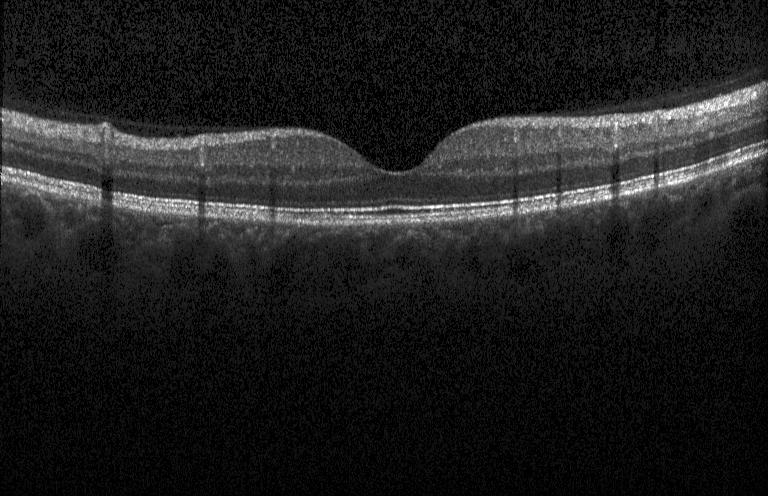

Macular OCT demonstrating no choroidal neovascularization, no diabetic macular edema, and no drusen.